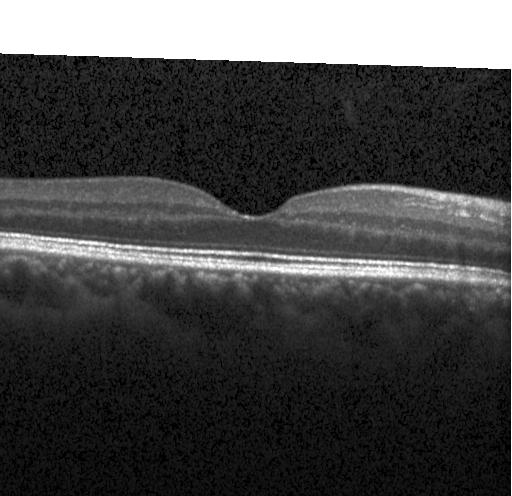 Diagnosis: neither choroidal neovascularization, diabetic macular edema, nor drusen.